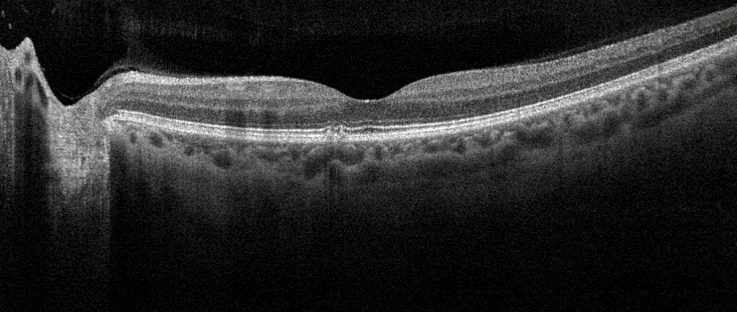 OCT B-scan. Instrument: Optovue Avanti RTVue XR. Fovea-centered. Finding: absence of AMD, DME, ERM, RAO, RVO, and vitreomacular interface disease.